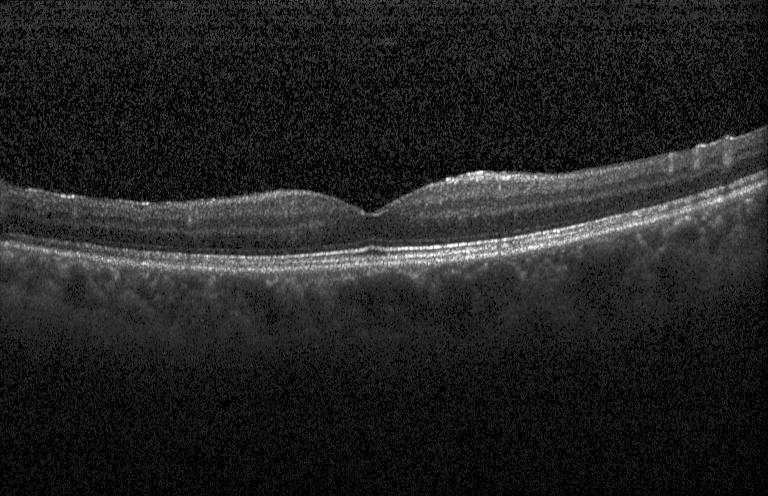
Through the macula, spectral-domain OCT, optical coherence tomography scan — Dx: no evidence of choroidal neovascularization, diabetic macular edema, or drusen.